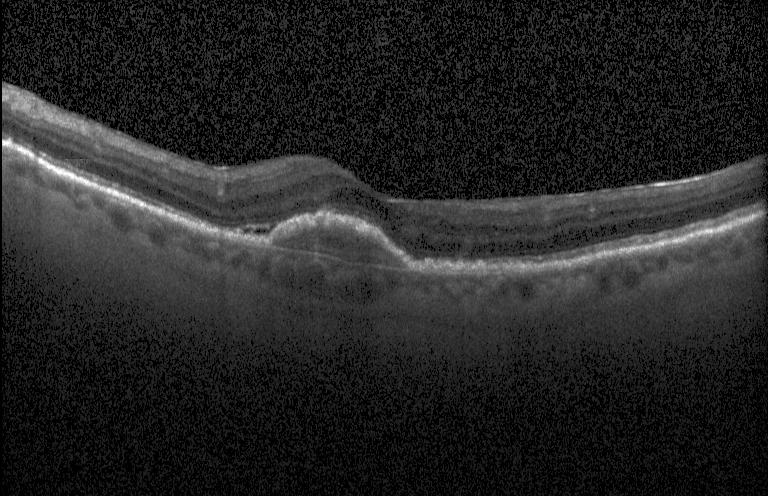

Optical coherence tomography scan; fovea-centered
Finding: a choroidal neovascular membrane.